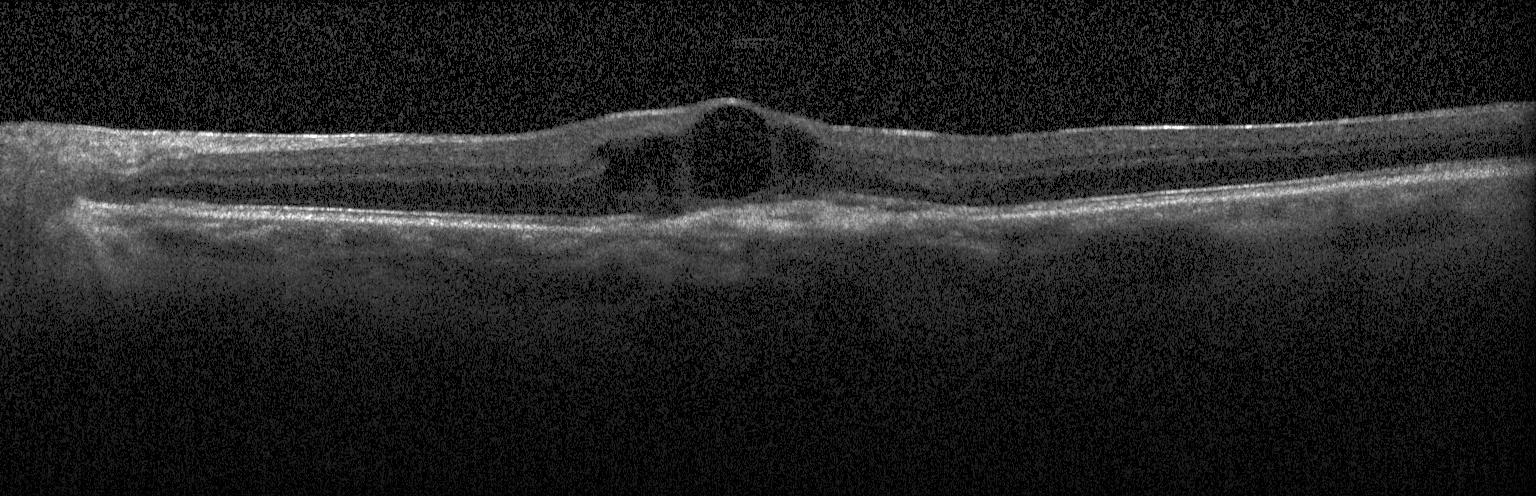

Retinal OCT B-scan — Impression: a choroidal neovascular membrane.